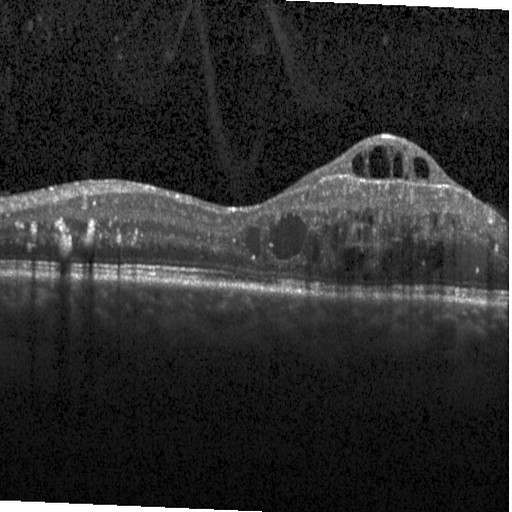 Macular scan; Heidelberg Spectralis; spectral-domain optical coherence tomography; retinal OCT B-scan.
Impression: diabetic macular edema (DME).